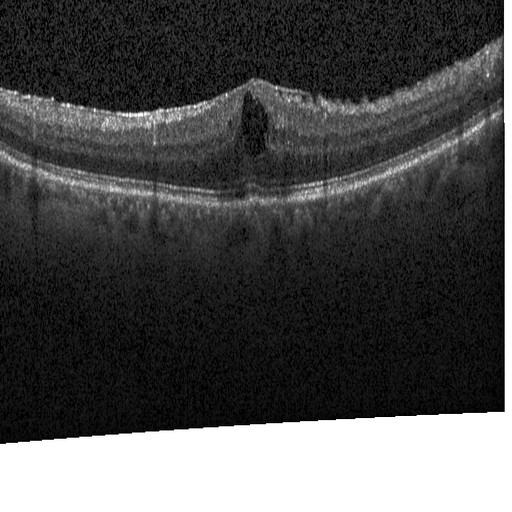 OCT B-scan. Diabetic macular edema (DME).